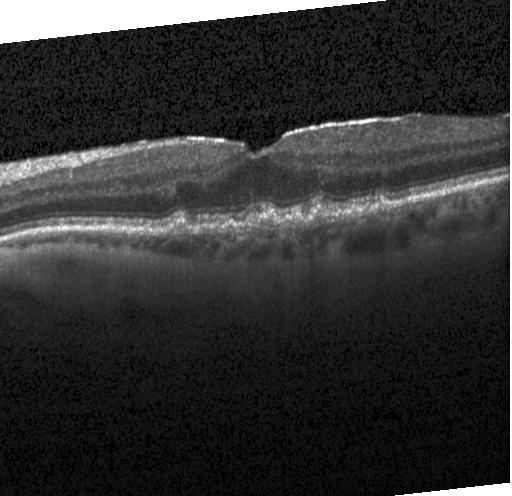

Optical coherence tomography scan, spectral-domain OCT, instrument: Heidelberg Spectralis. Assessment: sub-RPE drusenoid deposits.